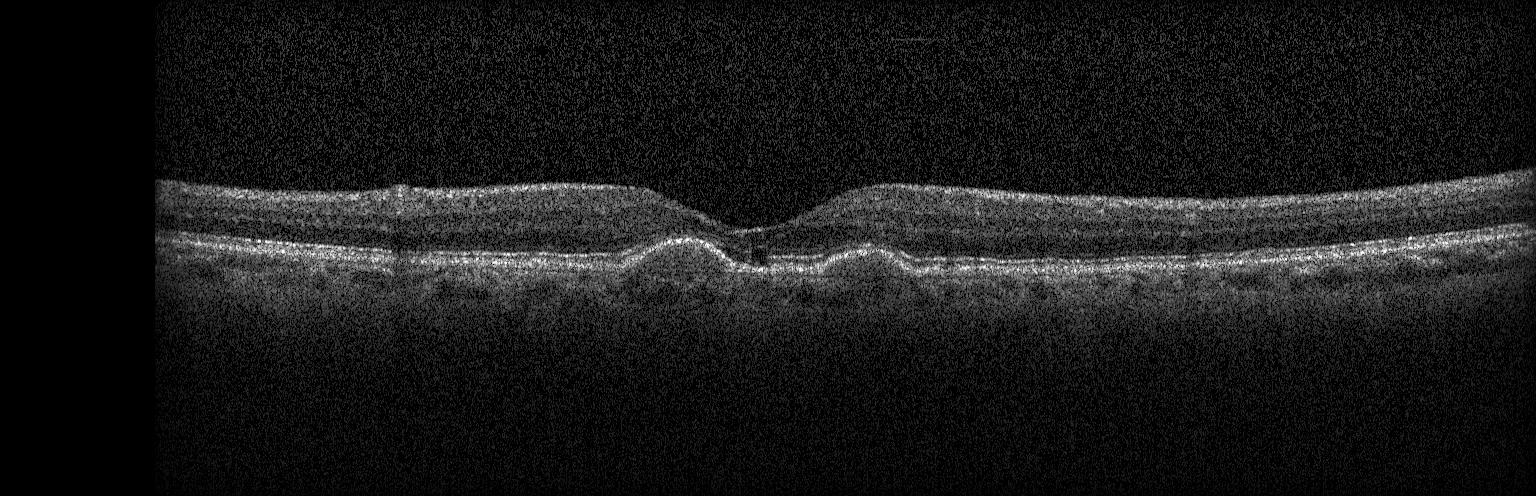

Fovea-centered; SD-OCT; optical coherence tomography scan; instrument: Heidelberg Spectralis
Diagnosis: multiple drusen.